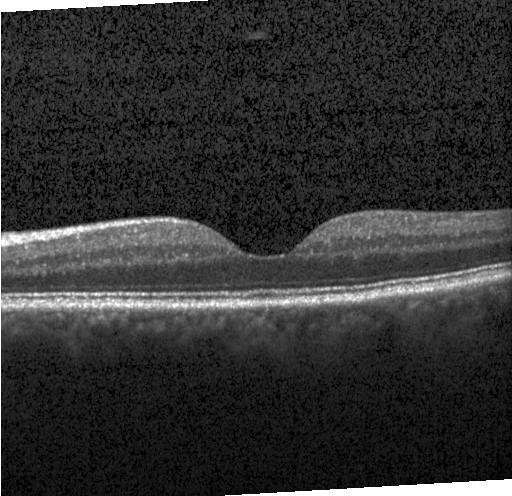

OCT finding: no choroidal neovascularization, diabetic macular edema, or drusen.